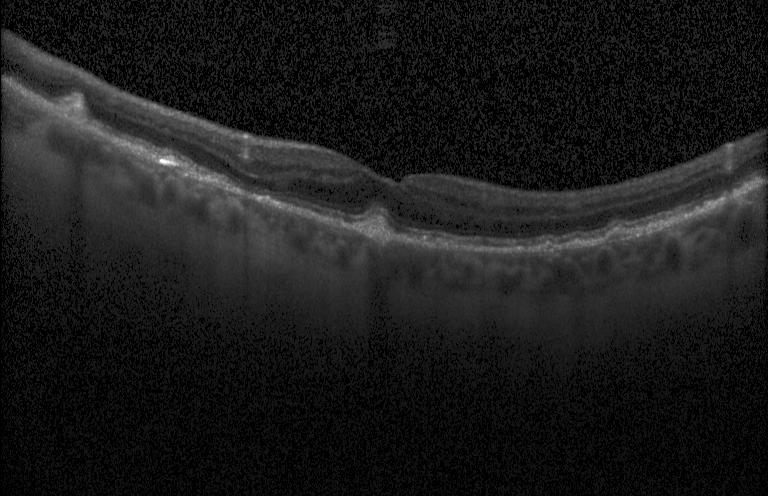
Retinal OCT B-scan. Instrument: Heidelberg Spectralis — Sub-RPE drusenoid deposits.